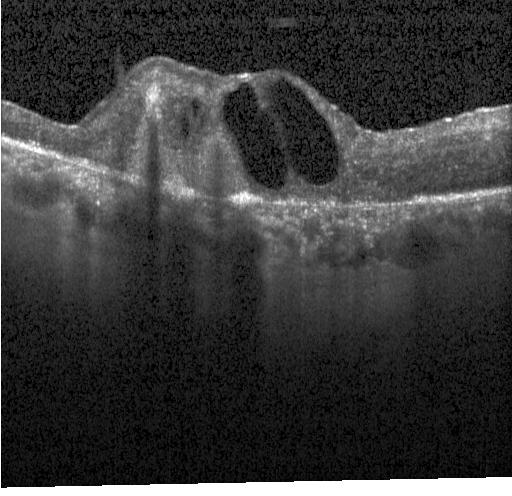

OCT B-scan; macular scan — The scan shows a choroidal neovascular membrane.